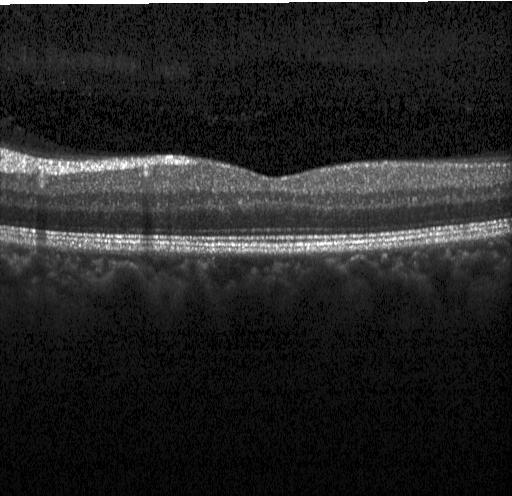 Retinal OCT cross-section showing neither choroidal neovascularization, diabetic macular edema, nor drusen.